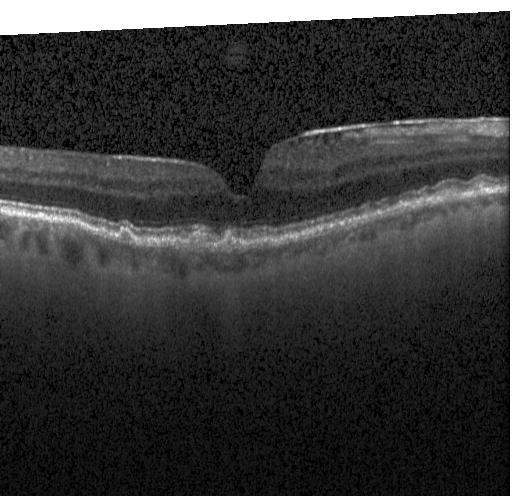
Diagnosis: drusen.